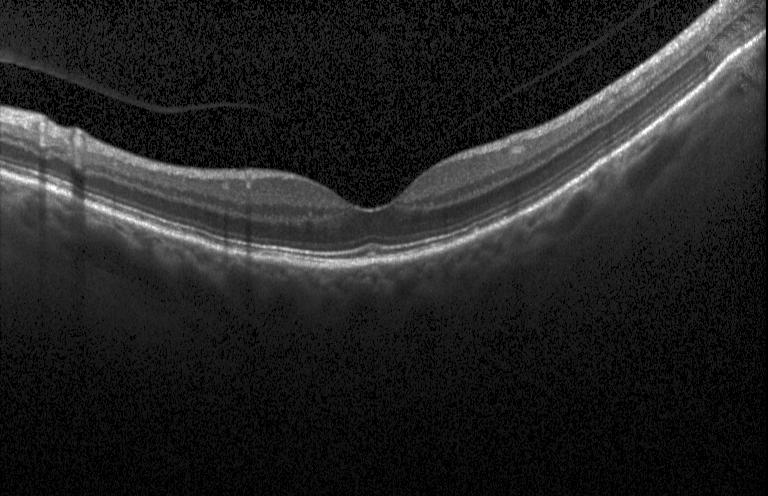 Assessment: no choroidal neovascularization, no diabetic macular edema, and no drusen.